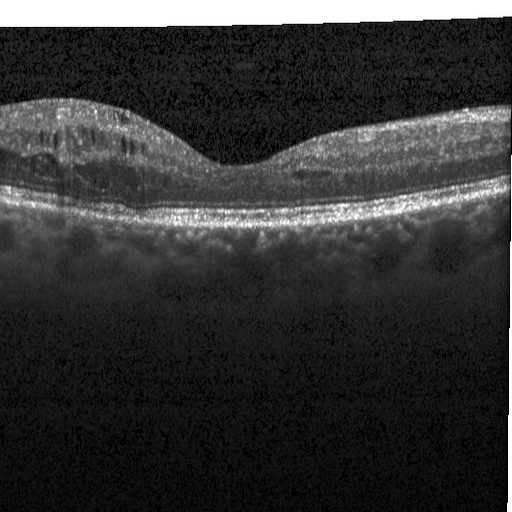
Heidelberg Spectralis OCT system. Fovea-centered. SD-OCT. OCT line scan — Diagnosis: diabetic macular edema.